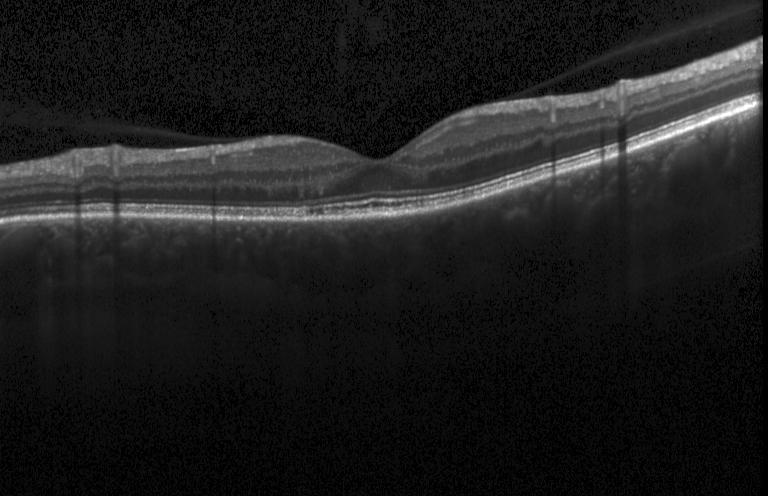
Assessment: no CNV, no DME, and no drusen.